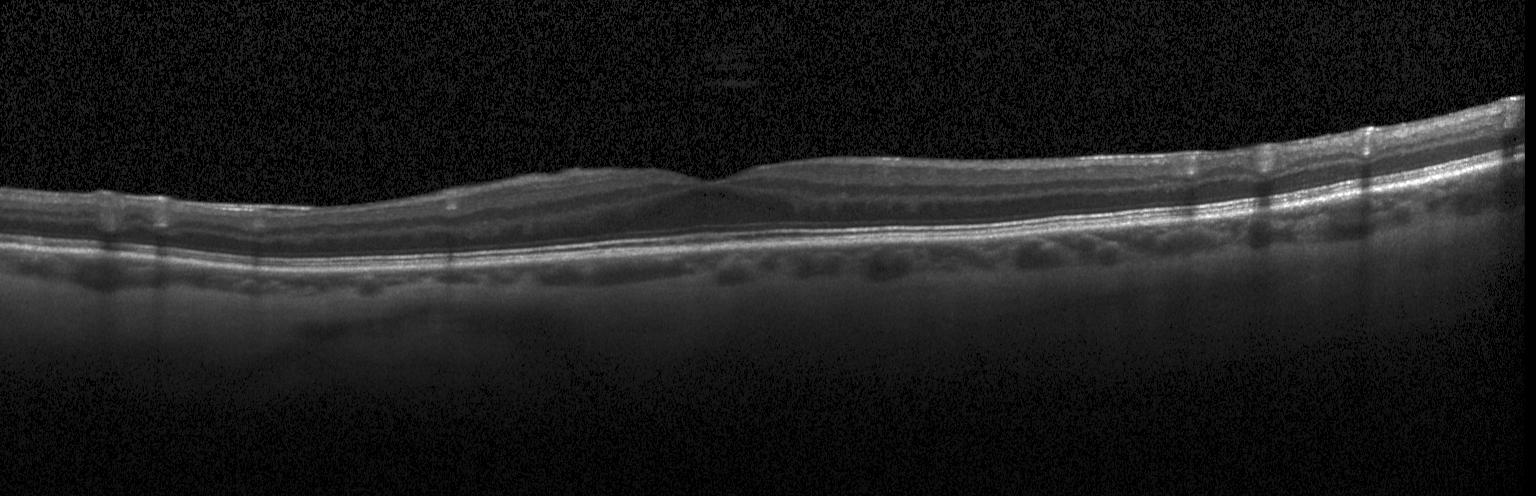 Heidelberg Spectralis, retinal OCT B-scan, horizontal scan through the fovea, spectral-domain optical coherence tomography. Macular OCT: neither choroidal neovascularization, diabetic macular edema, nor drusen.